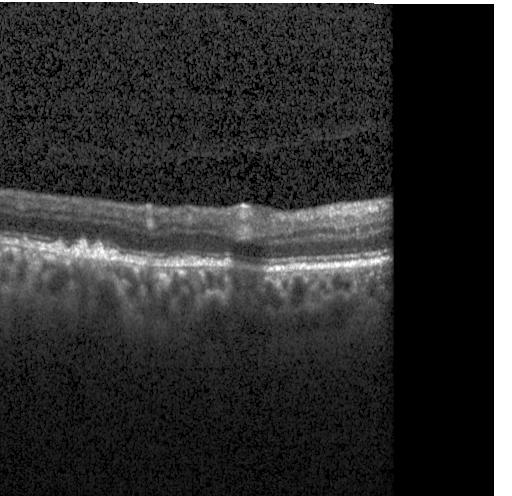 Finding: multiple drusen.